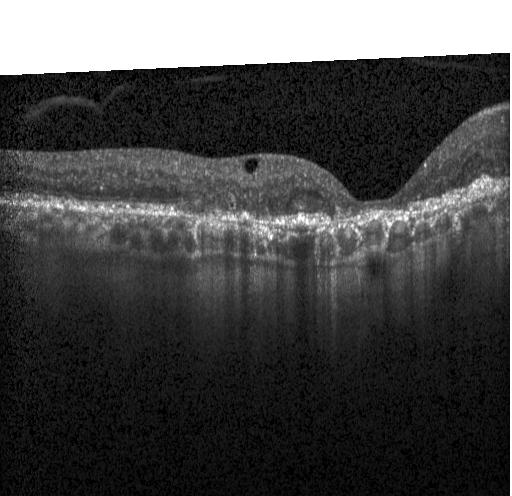 Optical coherence tomography B-scan · Heidelberg Spectralis OCT system · spectral-domain OCT · macular scan — Diagnosis: choroidal neovascularization.